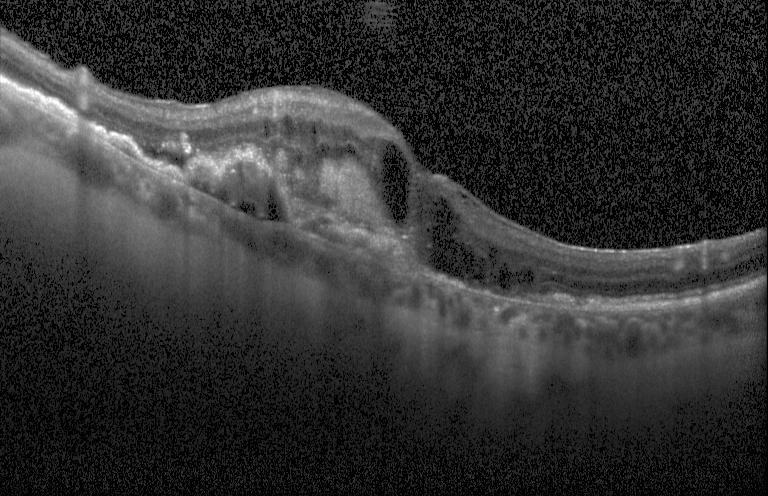

Assessment: a choroidal neovascular membrane.